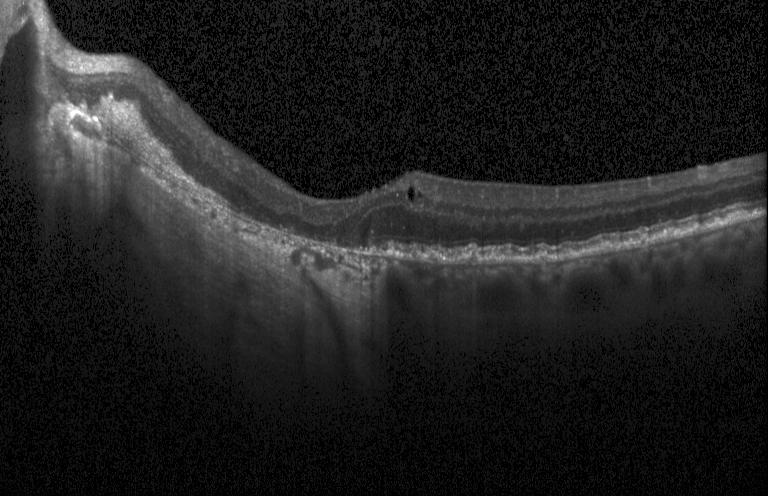

Spectral-domain optical coherence tomography. Retinal OCT B-scan. Heidelberg Spectralis. Centered on the fovea — Impression: a choroidal neovascular membrane.